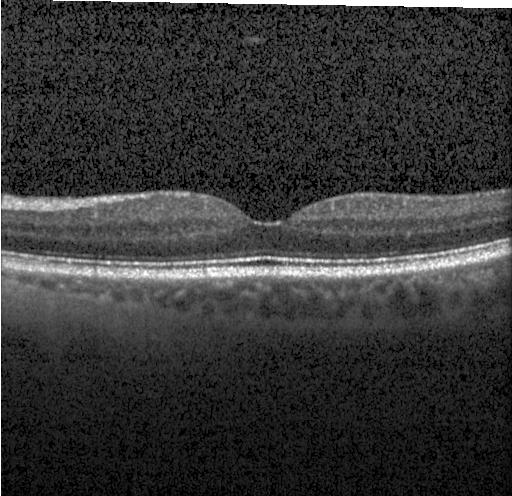

Diagnosis: no choroidal neovascularization, diabetic macular edema, or drusen.